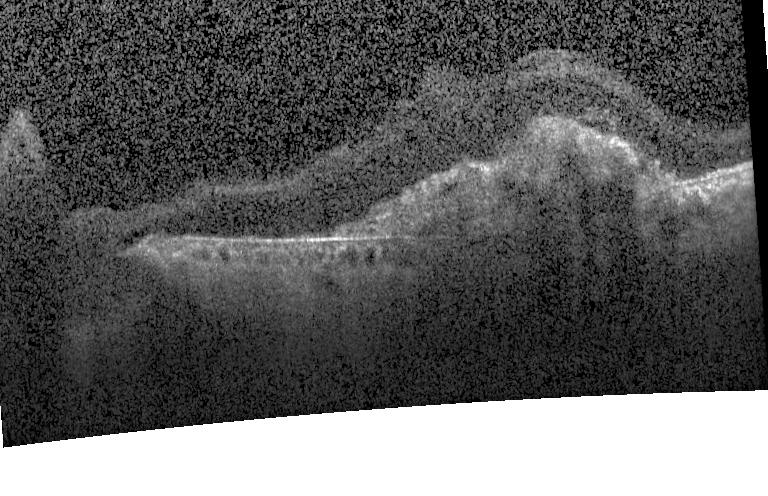 Retinal OCT B-scan
Finding: choroidal neovascularization.